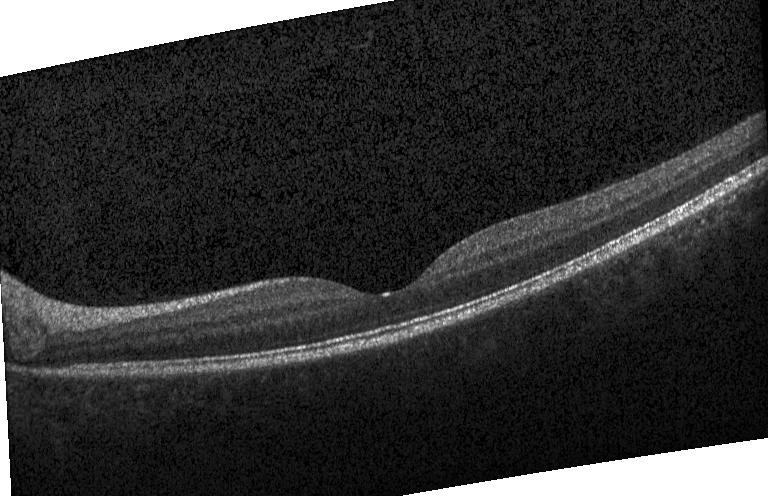
Heidelberg Spectralis · optical coherence tomography B-scan. Diagnosis: no choroidal neovascularization, diabetic macular edema, or drusen.